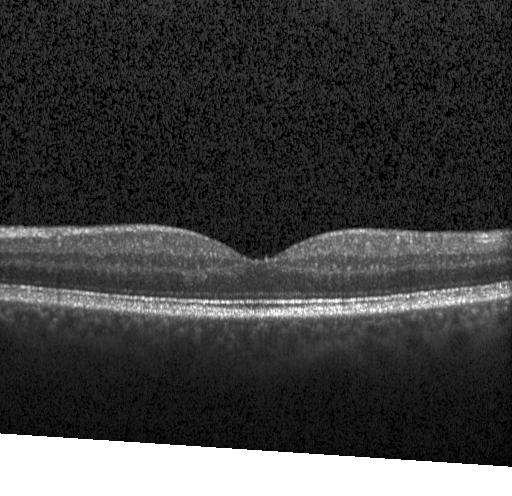
Retinal OCT B-scan. SD-OCT. Heidelberg Spectralis. Fovea-centered — Macular OCT: neither choroidal neovascularization, diabetic macular edema, nor drusen.